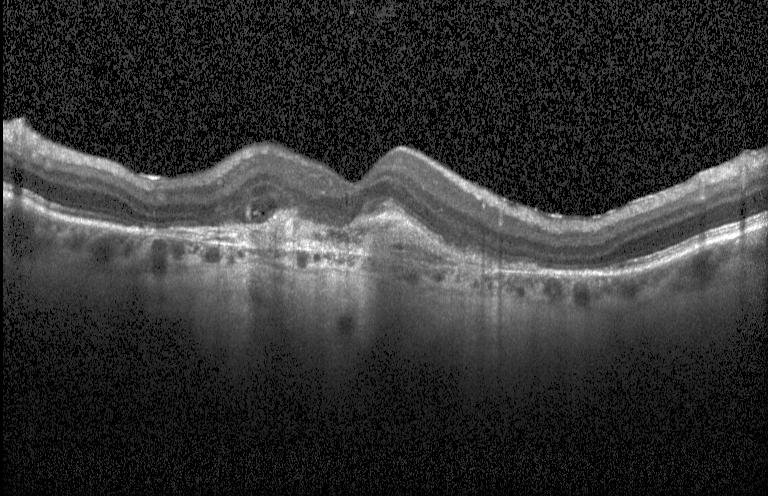 Heidelberg Spectralis, optical coherence tomography B-scan, fovea-centered
Diagnosis: a choroidal neovascular membrane.